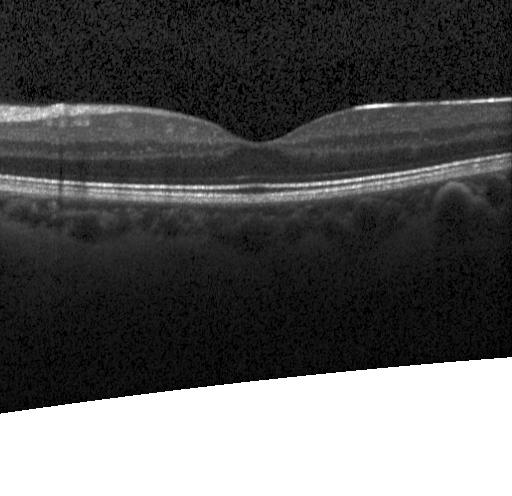

Retinal OCT cross-section showing neither CNV, DME, nor drusen.